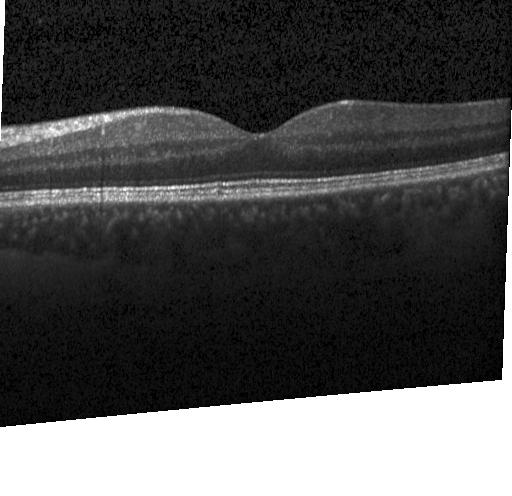

Heidelberg Spectralis OCT system, optical coherence tomography B-scan — Assessment: no choroidal neovascularization, no diabetic macular edema, and no drusen.